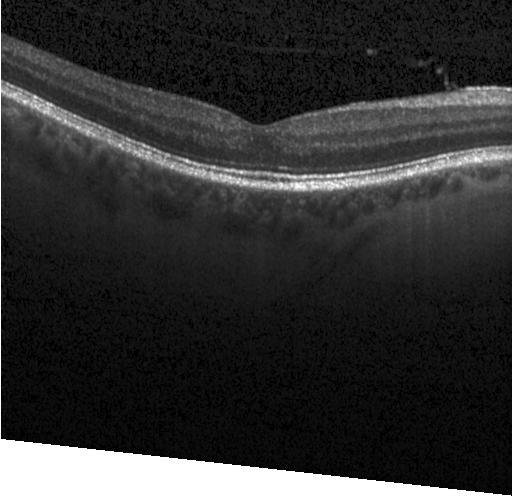 Spectral-domain OCT · optical coherence tomography B-scan. Impression: no CNV, DME, or drusen.